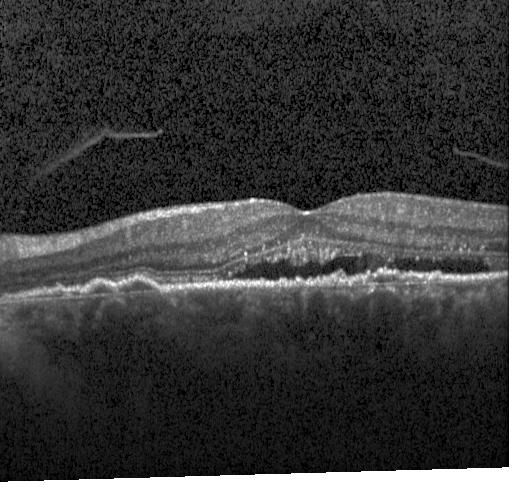 Retinal OCT cross-section.
Dx: a choroidal neovascular membrane.